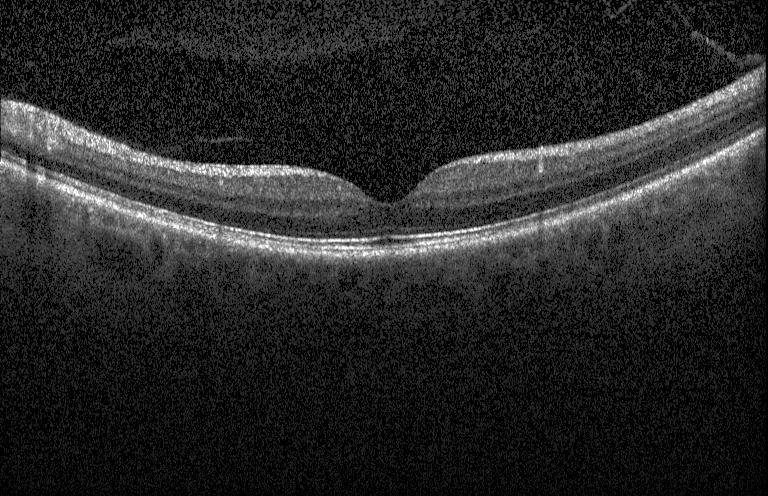
Finding: no CNV, no DME, and no drusen.